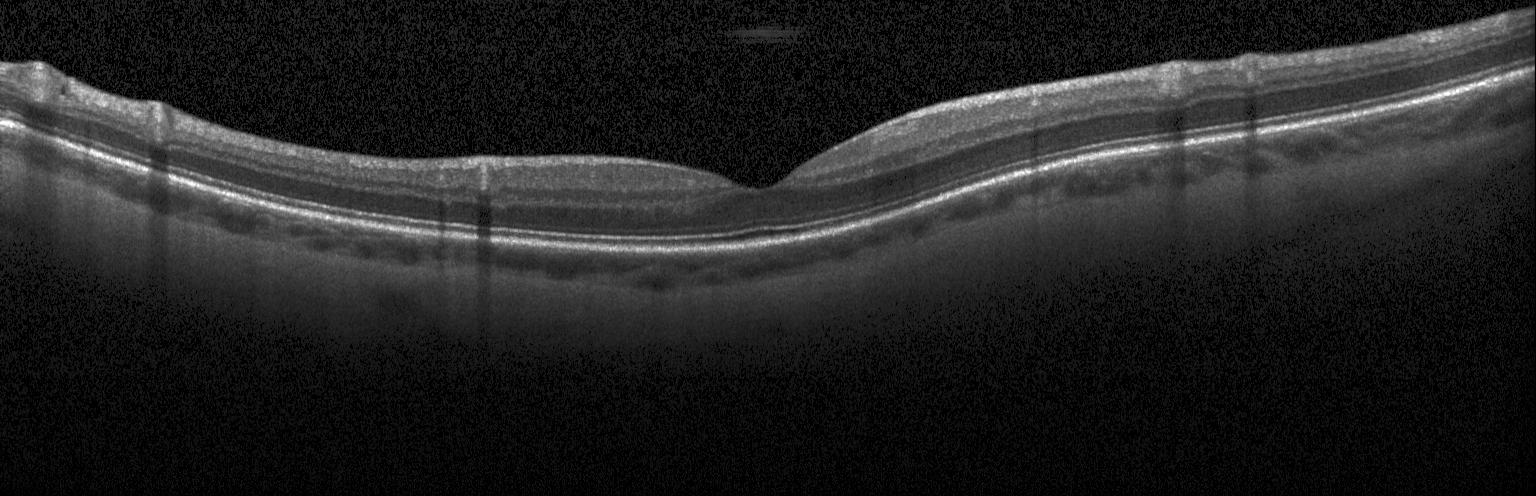

Macular OCT: no CNV, DME, or drusen.